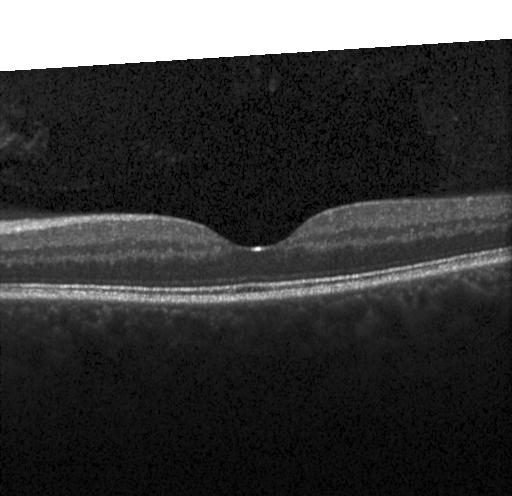 Macular scan · instrument: Heidelberg Spectralis · optical coherence tomography scan · spectral-domain optical coherence tomography
Macular OCT: no CNV, no DME, and no drusen.